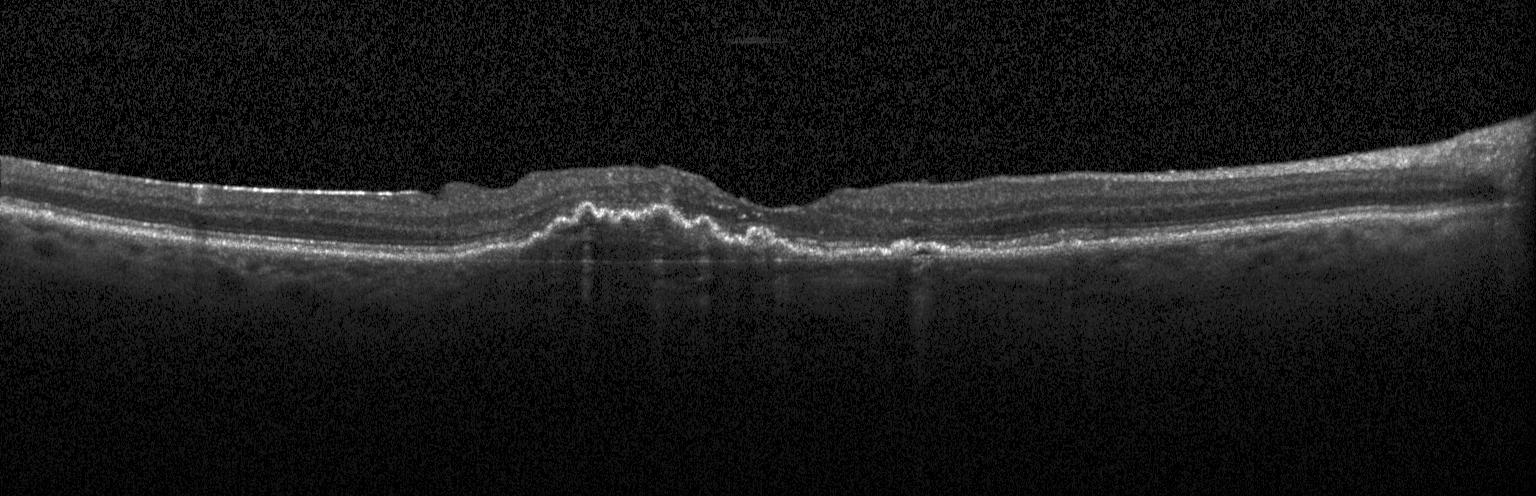 OCT B-scan; spectral-domain optical coherence tomography. Dx: CNV.